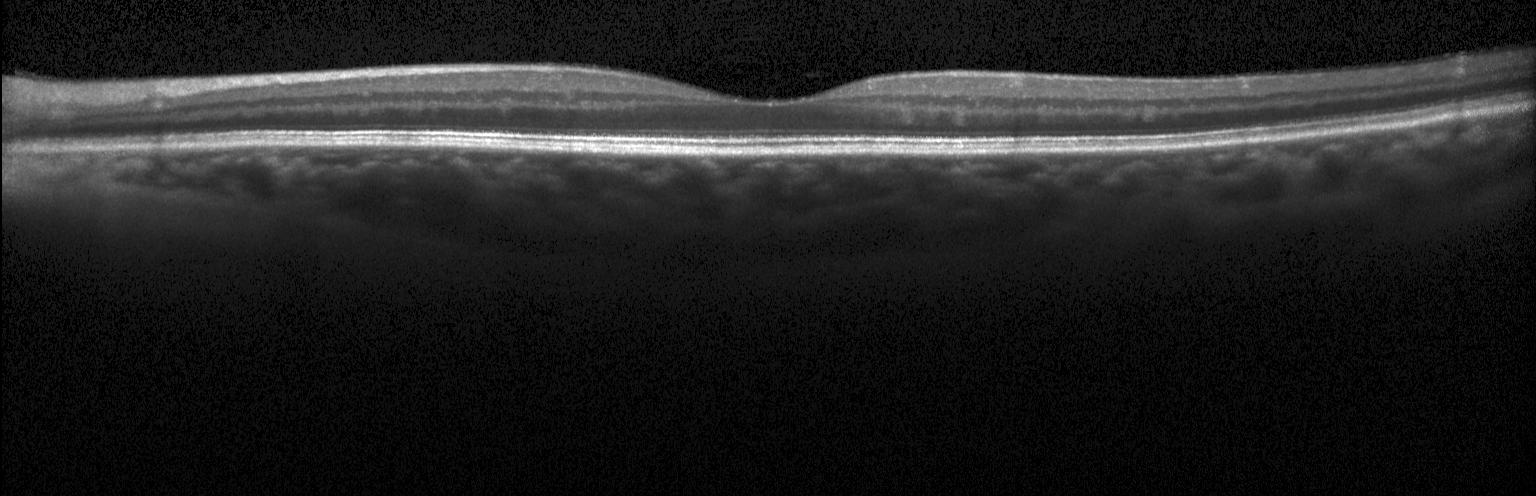

Neither choroidal neovascularization, diabetic macular edema, nor drusen.